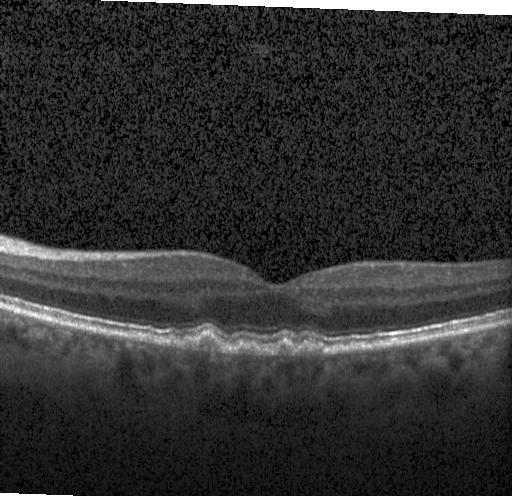
The scan shows multiple drusen.